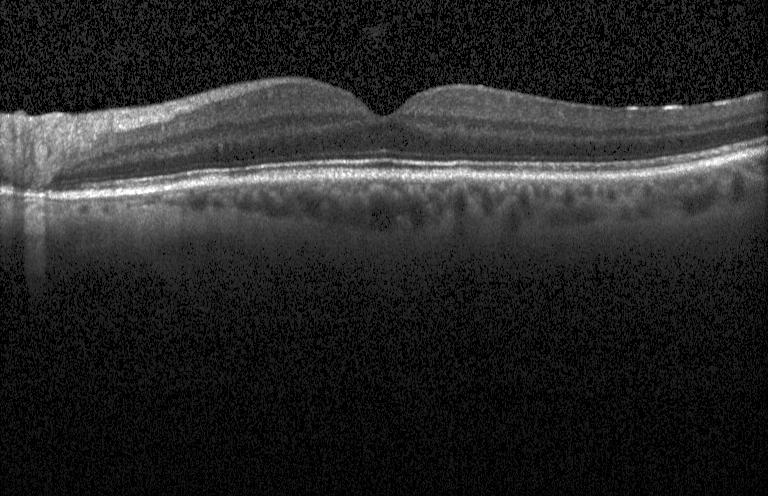

Optical coherence tomography scan. SD-OCT. Instrument: Heidelberg Spectralis. Horizontal scan through the fovea. Finding: no evidence of CNV, DME, or drusen.